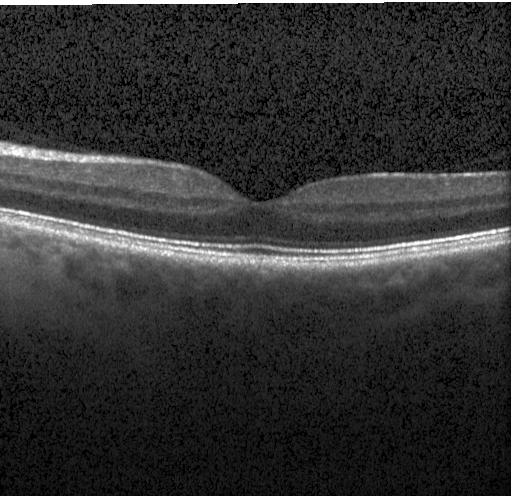 Optical coherence tomography scan. SD-OCT. Centered on the fovea
Finding: no choroidal neovascularization, no diabetic macular edema, and no drusen.